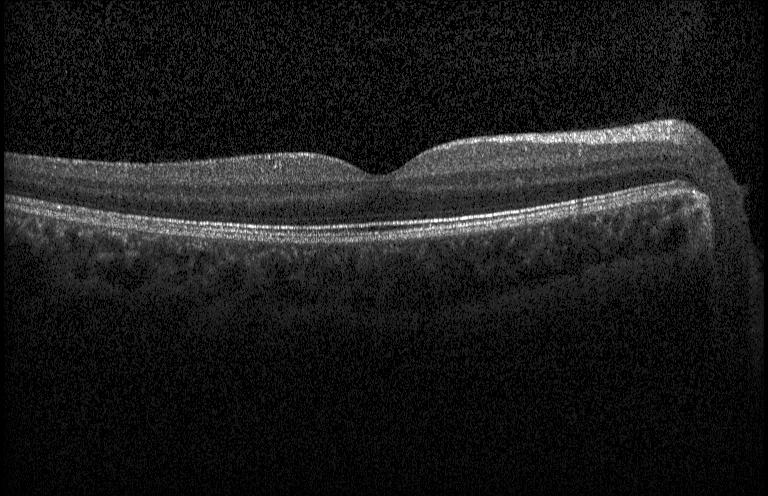 Finding: neither CNV, DME, nor drusen.